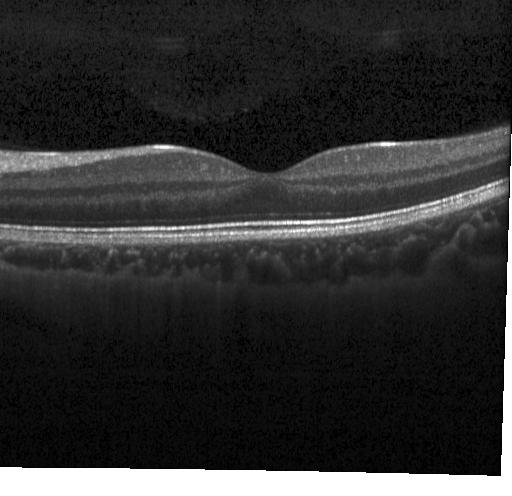
Macular scan; OCT B-scan; spectral-domain optical coherence tomography — Impression: neither choroidal neovascularization, diabetic macular edema, nor drusen.